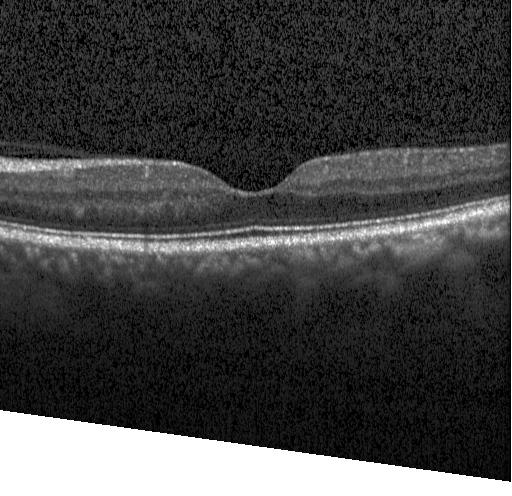

OCT B-scan.
No CNV, DME, or drusen.